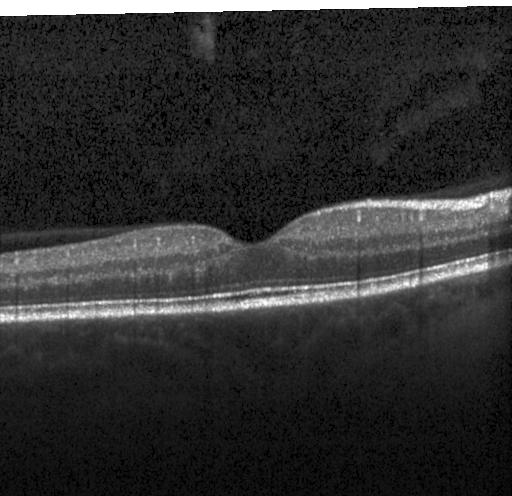 OCT line scan. Horizontal scan through the fovea
Diagnosis: neither CNV, DME, nor drusen.